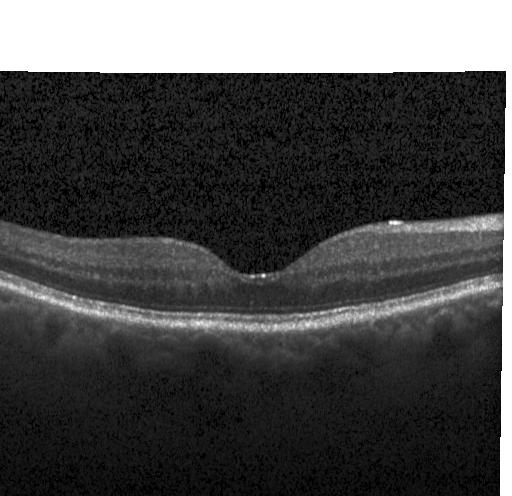
Macular OCT demonstrating no choroidal neovascularization, diabetic macular edema, or drusen.